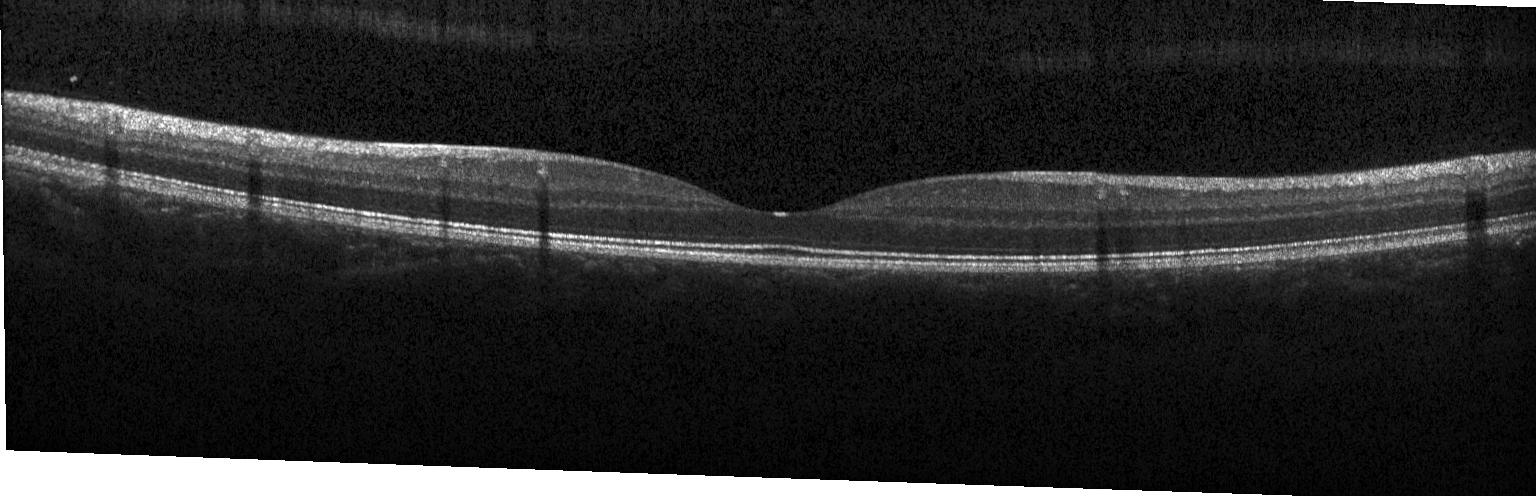 Impression: no choroidal neovascularization, no diabetic macular edema, and no drusen.